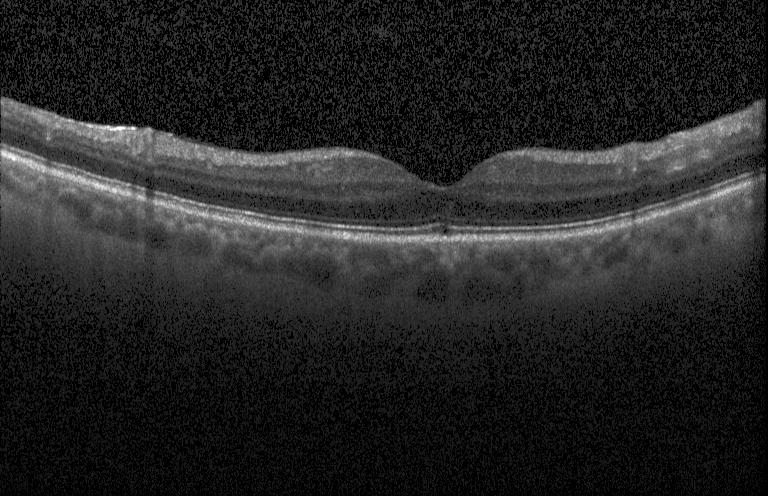
Heidelberg Spectralis OCT system · SD-OCT · optical coherence tomography scan · fovea-centered. Finding: no evidence of choroidal neovascularization, diabetic macular edema, or drusen.